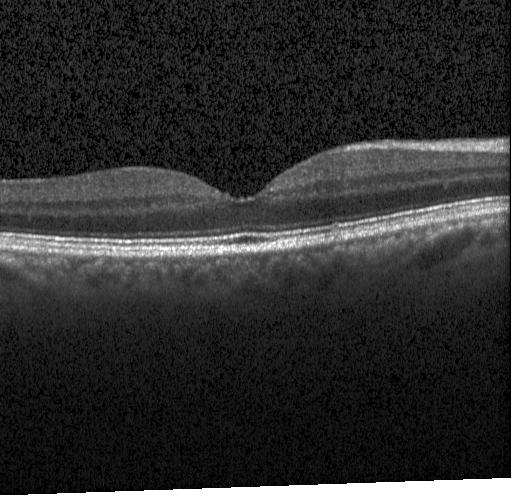

Fovea-centered. Retinal OCT B-scan. Acquired on a Heidelberg Spectralis — This B-scan demonstrates no evidence of choroidal neovascularization, diabetic macular edema, or drusen.